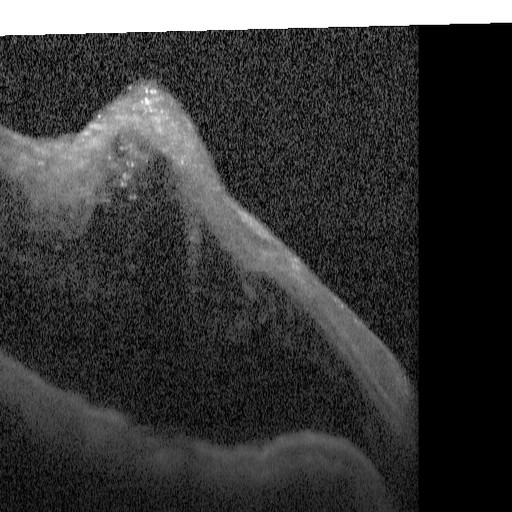
Optical coherence tomography scan. Dx: diabetic macular edema.